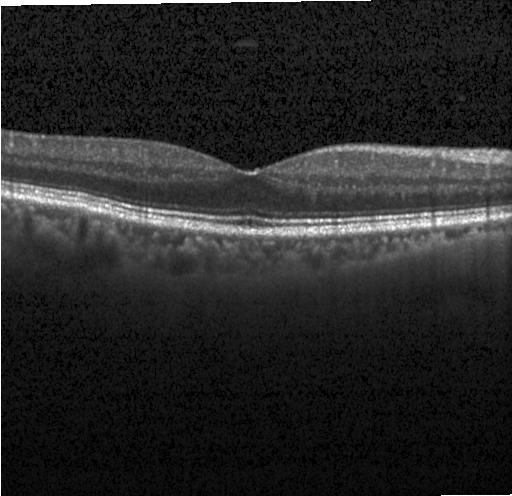
OCT finding: neither choroidal neovascularization, diabetic macular edema, nor drusen.